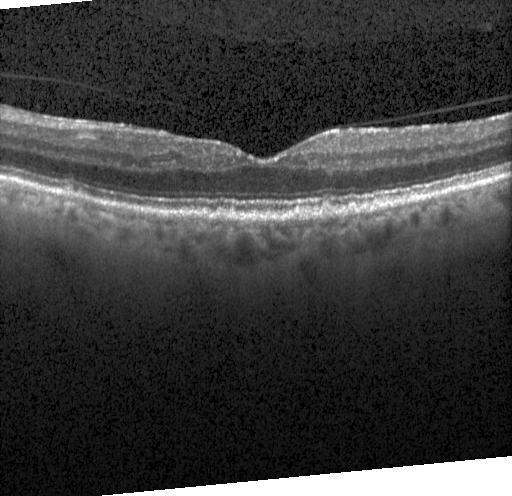
Retinal OCT cross-section showing drusen.